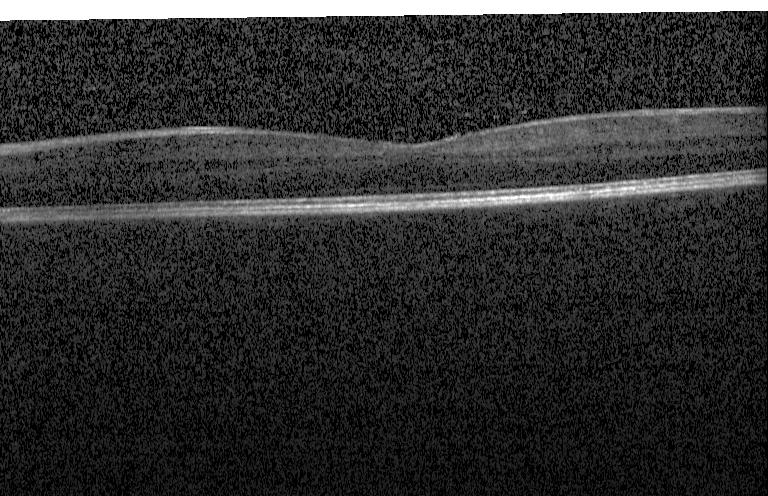
Through the macula · instrument: Heidelberg Spectralis · retinal OCT cross-section · spectral-domain OCT.
Diagnosis: no evidence of CNV, DME, or drusen.